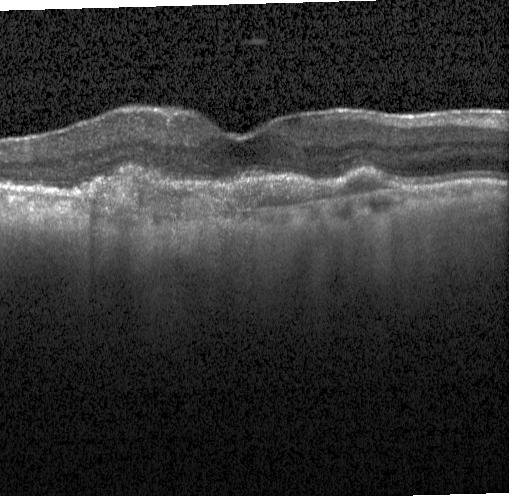
Heidelberg Spectralis OCT system, SD-OCT, optical coherence tomography scan, fovea-centered
Diagnosis: a choroidal neovascular membrane.